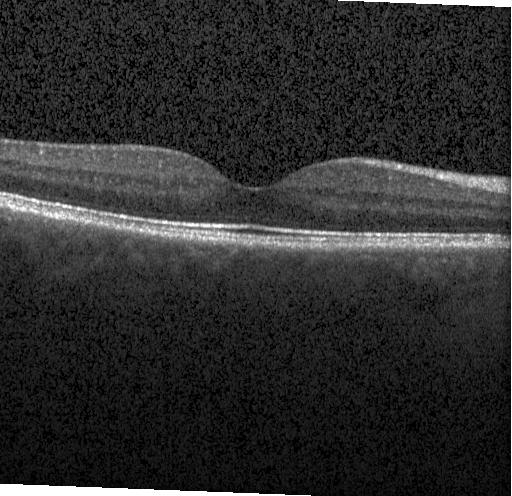

Finding: no evidence of choroidal neovascularization, diabetic macular edema, or drusen.